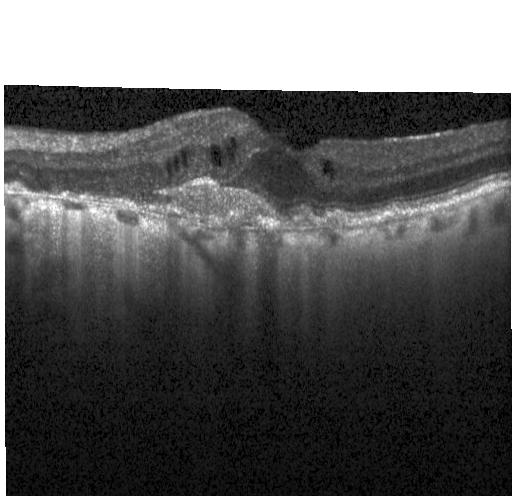
Retinal OCT B-scan
Finding: choroidal neovascularization (CNV).